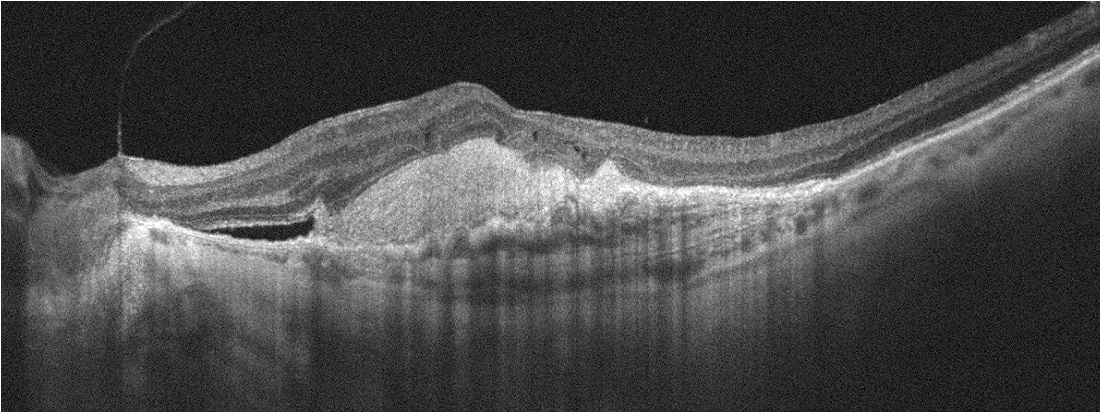 Finding: age-related macular degeneration (AMD).